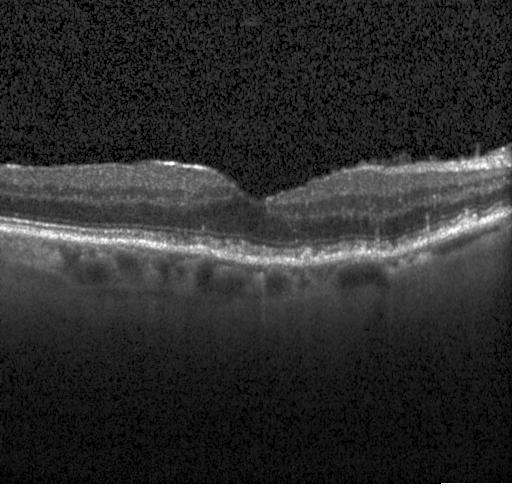 Dx: sub-RPE drusenoid deposits.